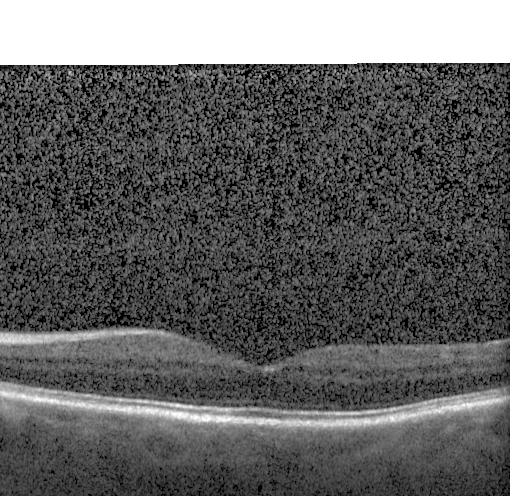 Horizontal scan through the fovea · optical coherence tomography scan
Impression: neither CNV, DME, nor drusen.